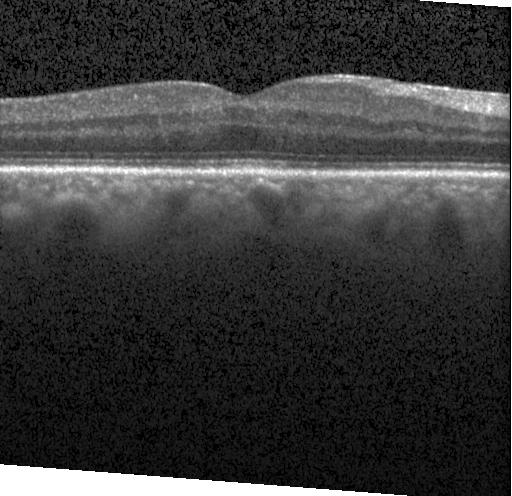
OCT line scan · SD-OCT — Finding: no evidence of choroidal neovascularization, diabetic macular edema, or drusen.